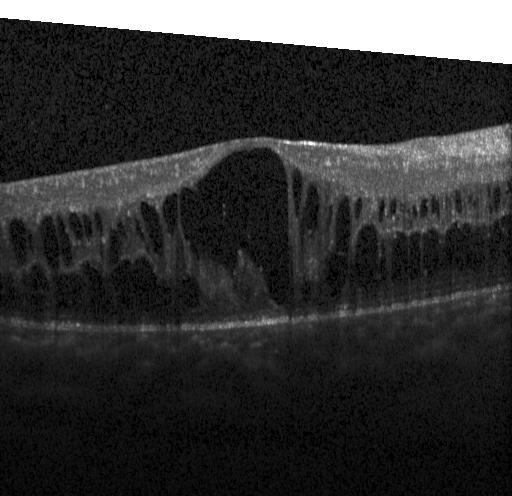 Spectral-domain optical coherence tomography; Heidelberg Spectralis; OCT line scan
DME.